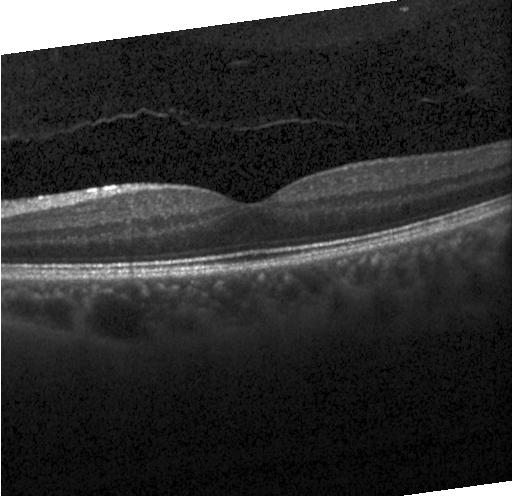
Dx: no evidence of choroidal neovascularization, diabetic macular edema, or drusen.